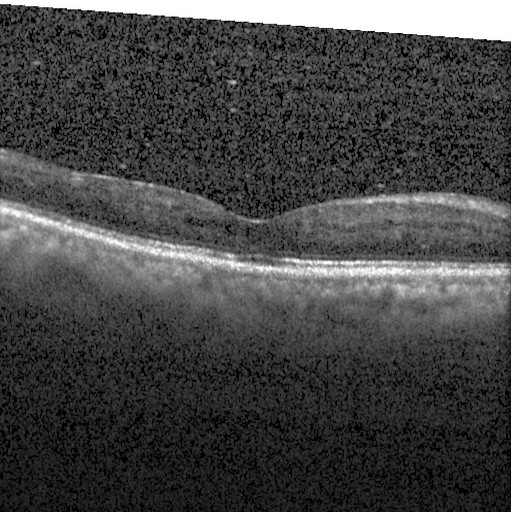 OCT B-scan showing diabetic macular edema.